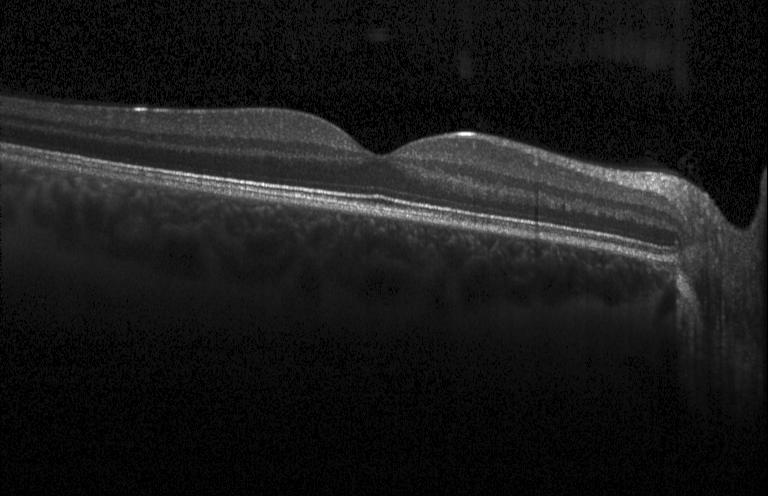 OCT B-scan. Centered on the fovea. Acquired on a Heidelberg Spectralis. Finding: no CNV, no DME, and no drusen.